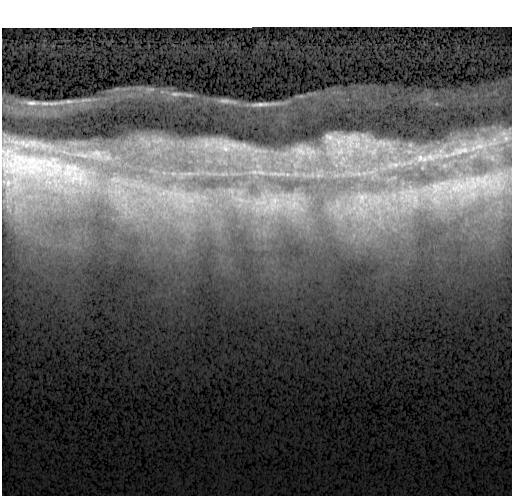

Horizontal scan through the fovea. Retinal OCT B-scan. Spectral-domain OCT — Impression: choroidal neovascularization (CNV).